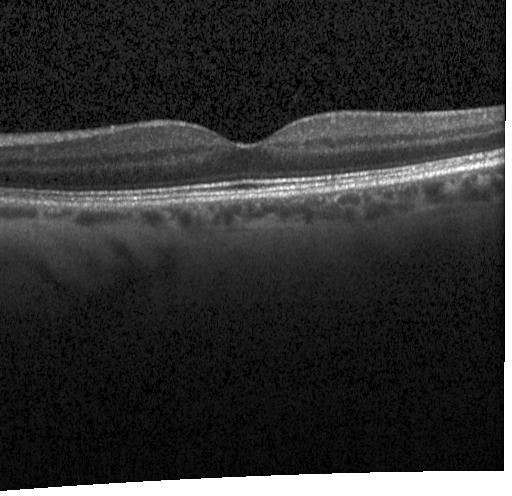

Centered on the fovea · retinal OCT cross-section — Finding: no choroidal neovascularization, no diabetic macular edema, and no drusen.